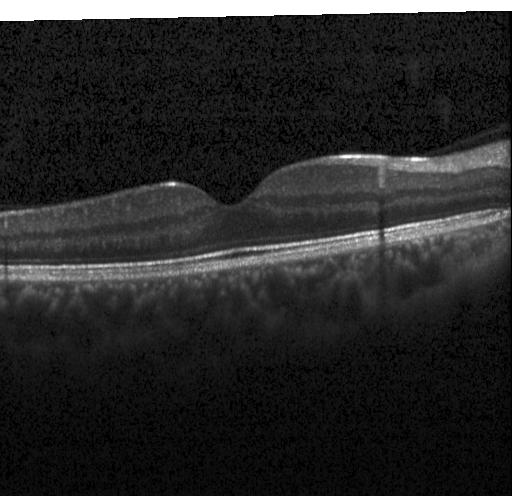
OCT B-scan showing no evidence of CNV, DME, or drusen.